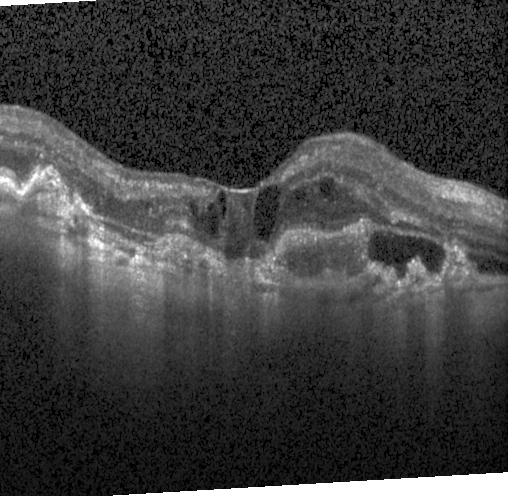
Choroidal neovascularization.